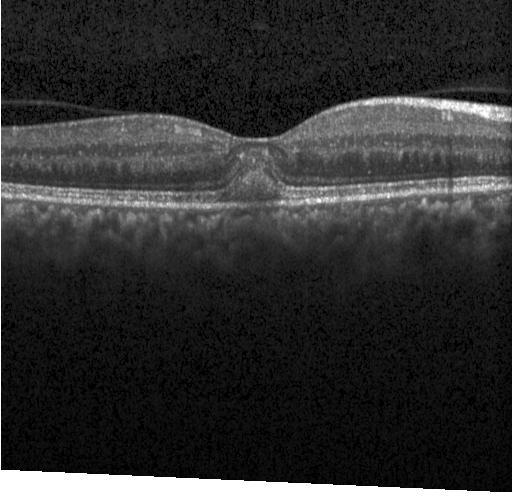 Retinal OCT cross-section. OCT finding: CNV.